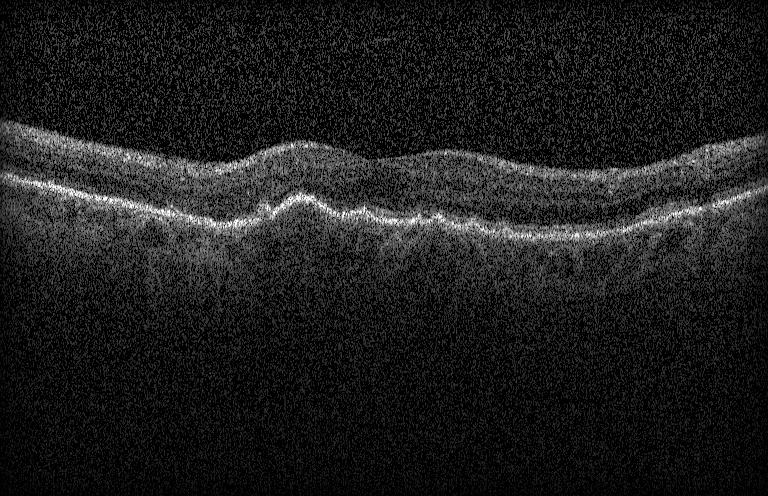 Diagnosis: a choroidal neovascular membrane.